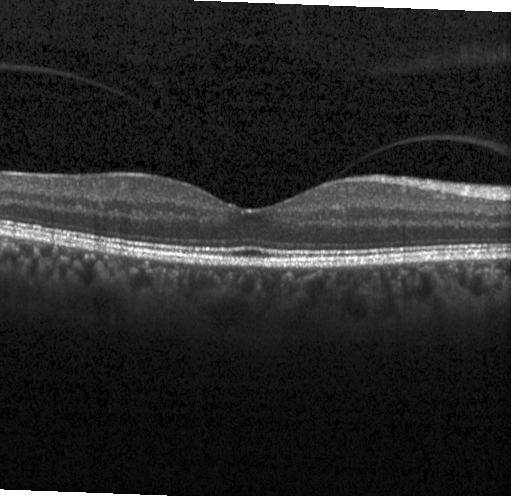

OCT line scan; horizontal scan through the fovea — Assessment: no CNV, no DME, and no drusen.